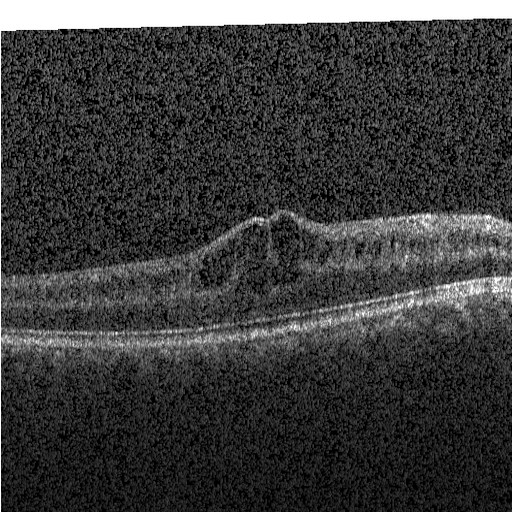 Centered on the fovea, spectral-domain OCT, optical coherence tomography B-scan, Heidelberg Spectralis. This B-scan demonstrates diabetic macular edema (DME).